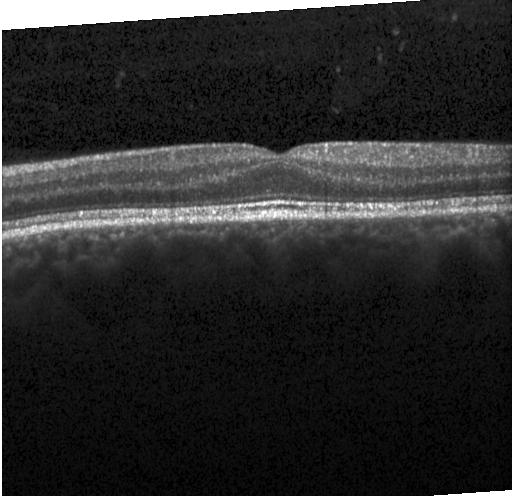 Retinal OCT cross-section · SD-OCT · acquired on a Heidelberg Spectralis · macular scan — Impression: no choroidal neovascularization, diabetic macular edema, or drusen.